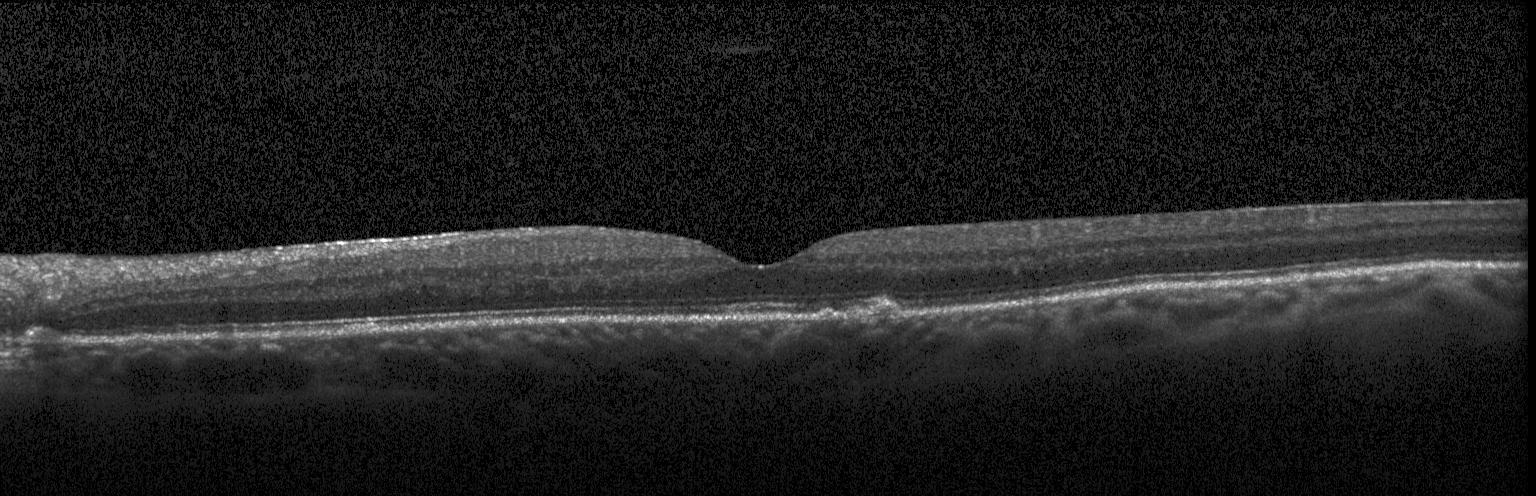 Optical coherence tomography B-scan. Dx: drusen.